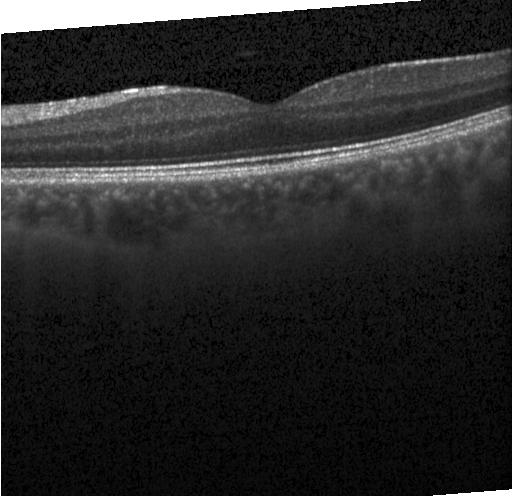
Retinal OCT B-scan
Diagnosis: no choroidal neovascularization, diabetic macular edema, or drusen.